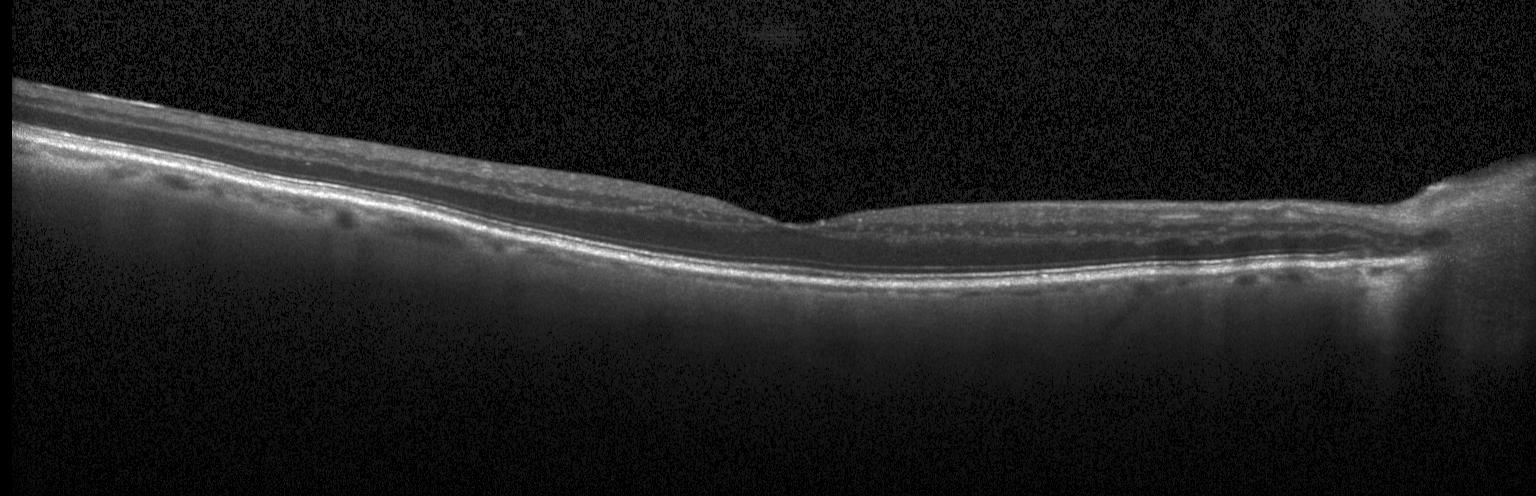

OCT B-scan showing no choroidal neovascularization, diabetic macular edema, or drusen.